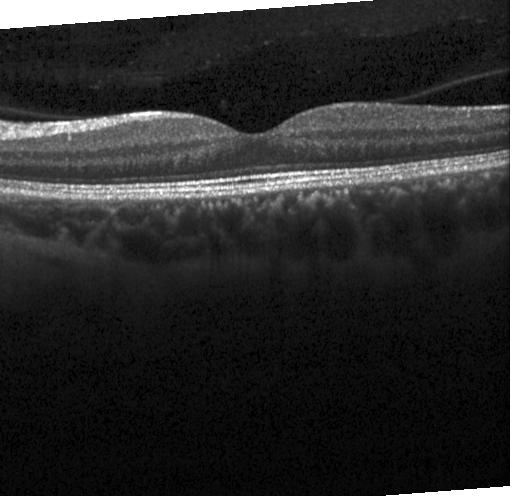
Optical coherence tomography B-scan — Macular OCT: no CNV, DME, or drusen.